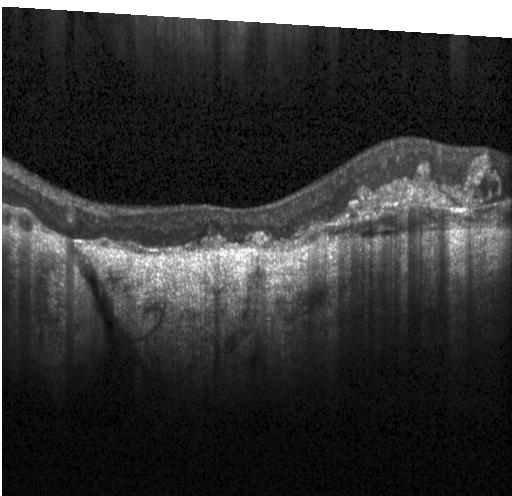 Diagnosis: choroidal neovascularization.